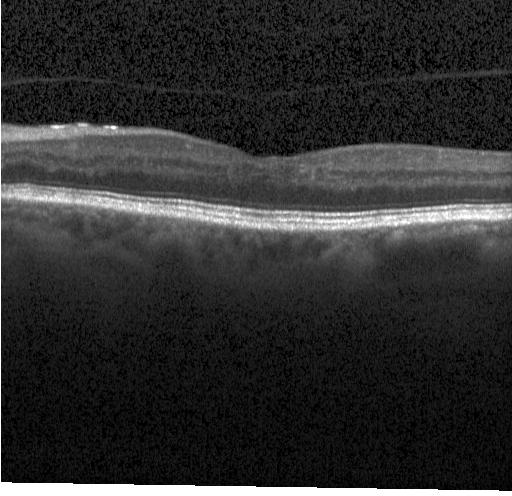

Through the macula. OCT B-scan. No evidence of CNV, DME, or drusen.